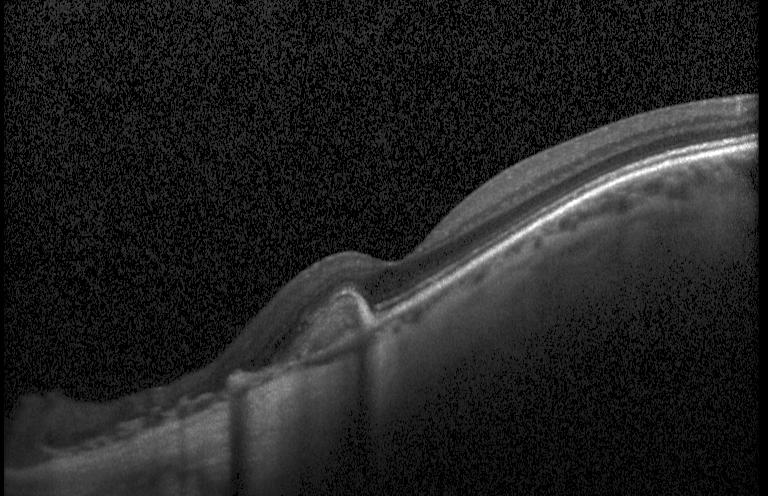 The scan shows choroidal neovascularization.